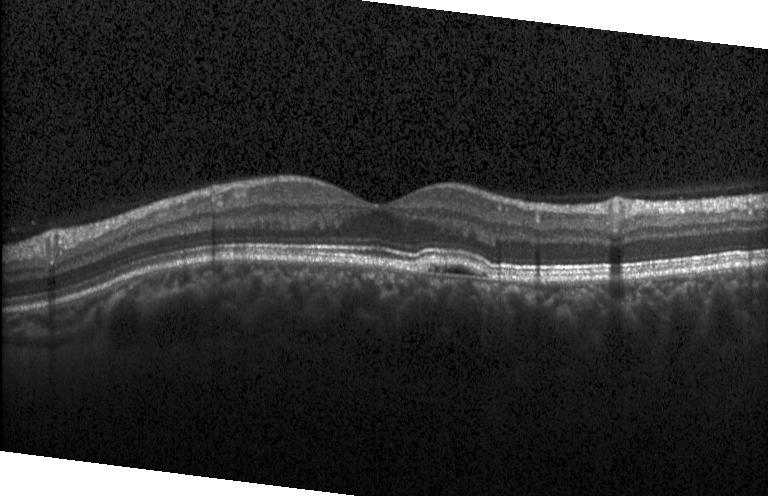 OCT B-scan — The scan shows a choroidal neovascular membrane.